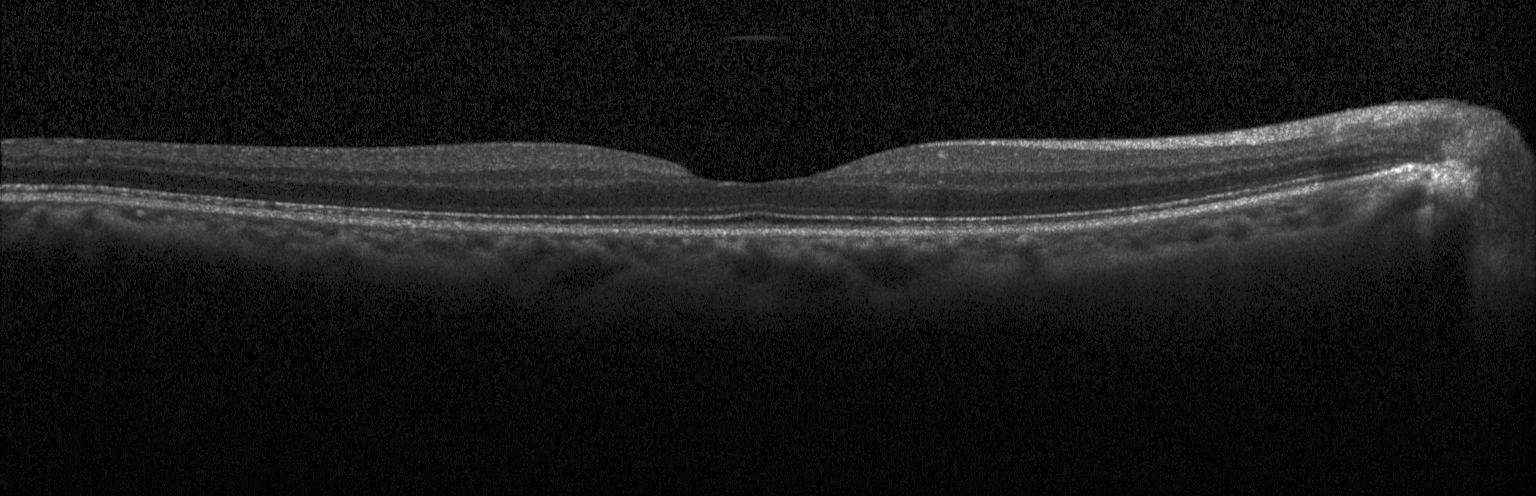 OCT line scan · SD-OCT · Heidelberg Spectralis OCT system · macular scan.
This B-scan demonstrates neither CNV, DME, nor drusen.